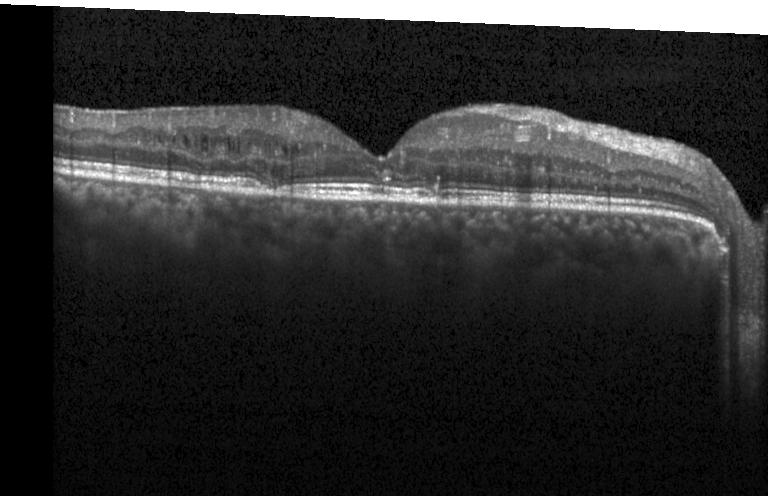
Diagnosis: diabetic macular edema (DME).